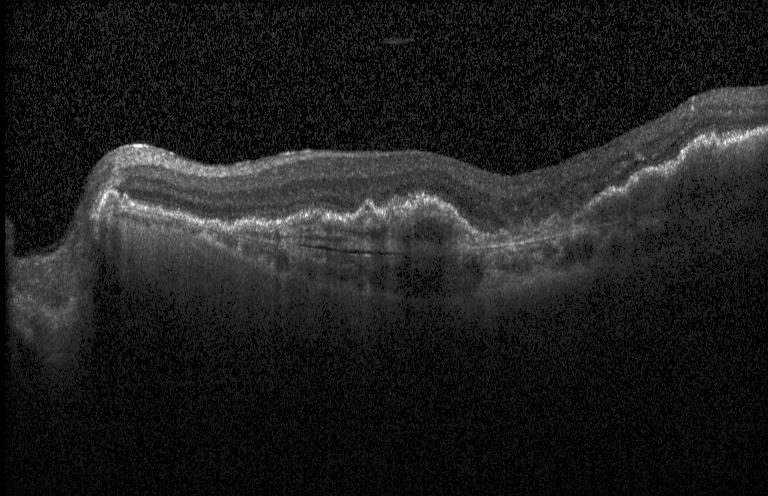 Choroidal neovascularization.